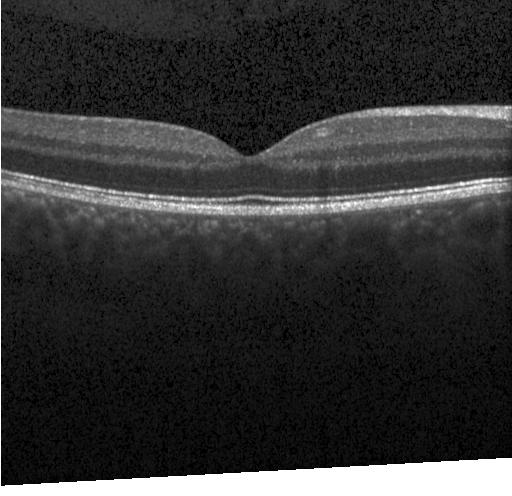 SD-OCT, instrument: Heidelberg Spectralis, through the macula, OCT B-scan
Assessment: neither CNV, DME, nor drusen.